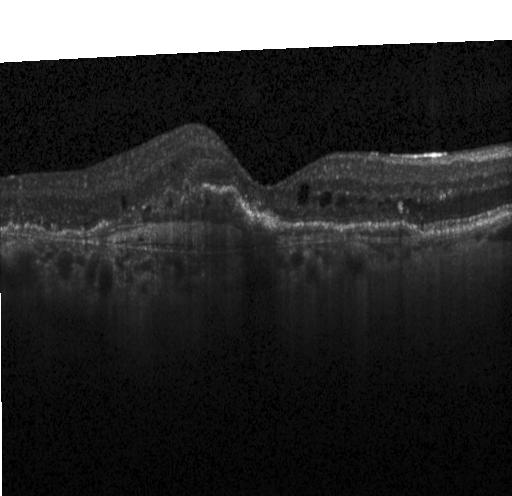

OCT line scan. Instrument: Heidelberg Spectralis
Diagnosis: a choroidal neovascular membrane.